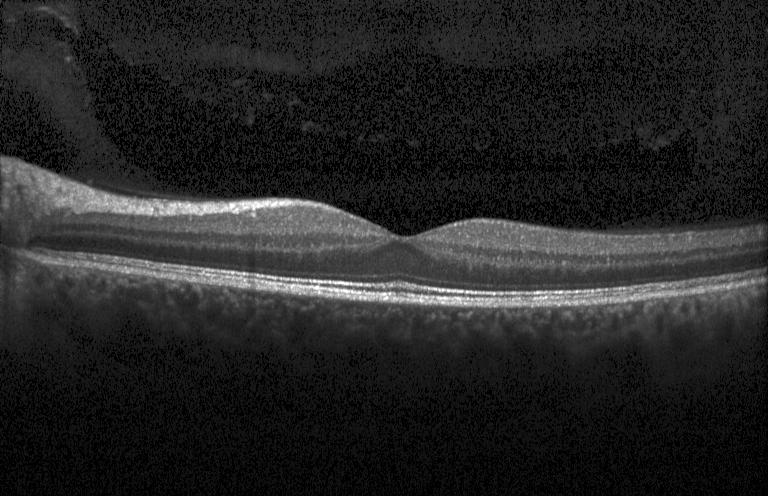 Spectral-domain optical coherence tomography. Retinal OCT B-scan. Centered on the fovea. Acquired on a Heidelberg Spectralis — Assessment: no evidence of choroidal neovascularization, diabetic macular edema, or drusen.